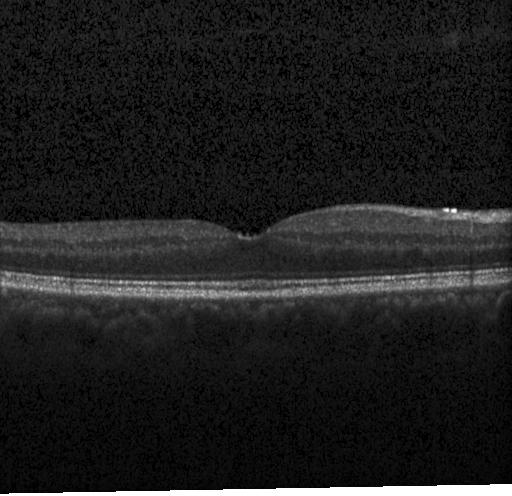
Centered on the fovea; OCT B-scan; spectral-domain OCT; Heidelberg Spectralis OCT system — Diagnosis: neither CNV, DME, nor drusen.